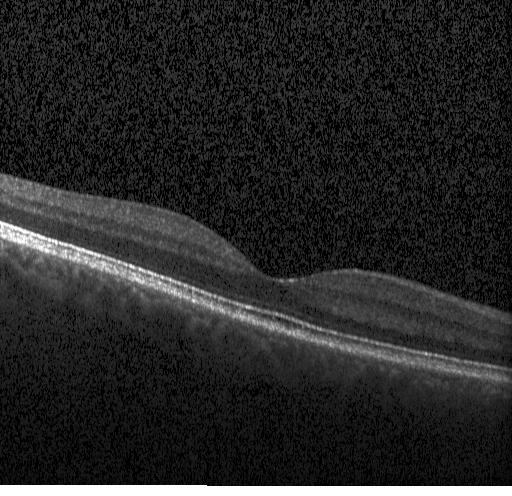 Macular OCT demonstrating neither CNV, DME, nor drusen.